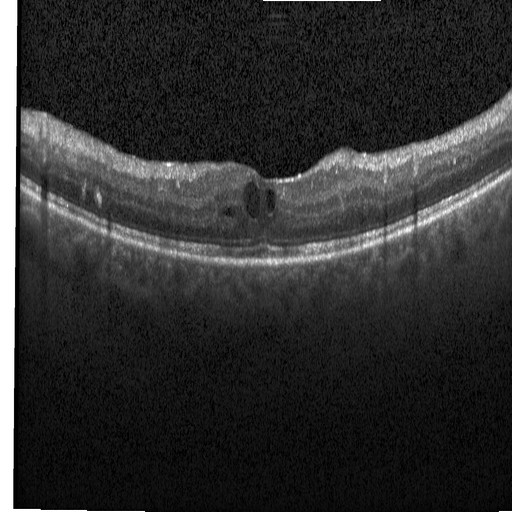
Diabetic macular edema.